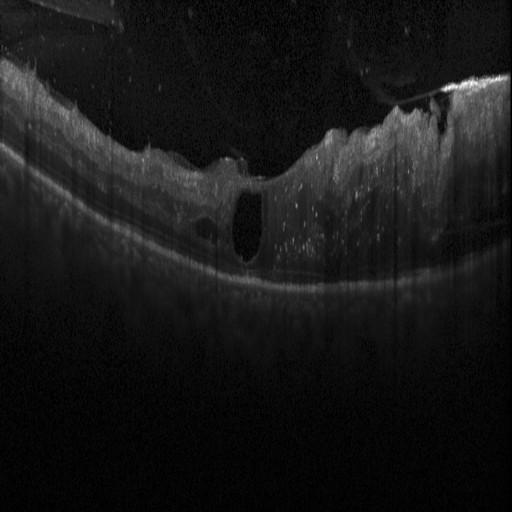 OCT finding: DME.